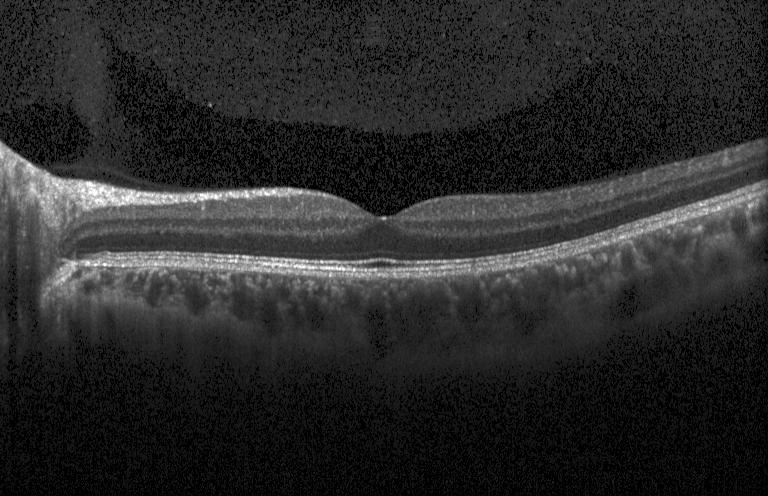
Macular OCT: no choroidal neovascularization, diabetic macular edema, or drusen.